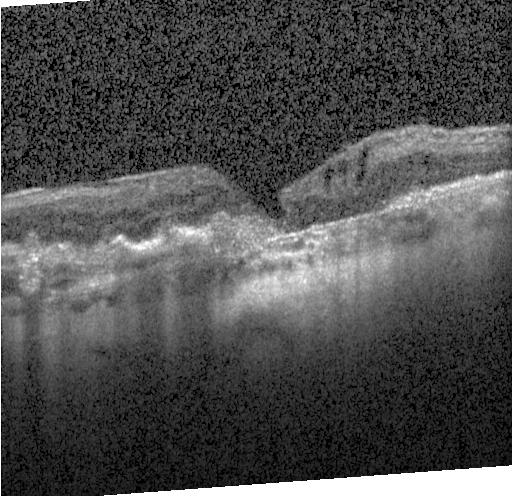

OCT B-scan showing CNV.